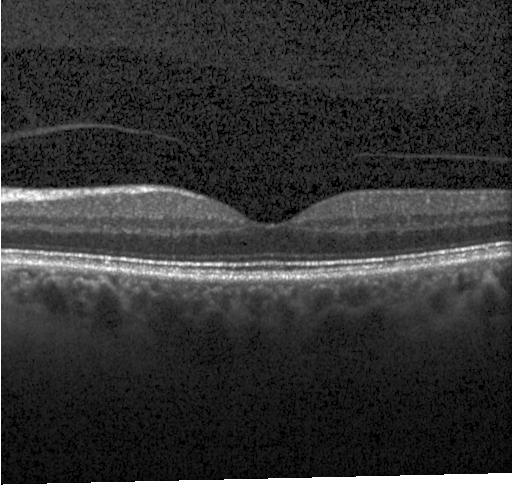
Heidelberg Spectralis; spectral-domain OCT; fovea-centered; OCT B-scan.
Assessment: no choroidal neovascularization, no diabetic macular edema, and no drusen.